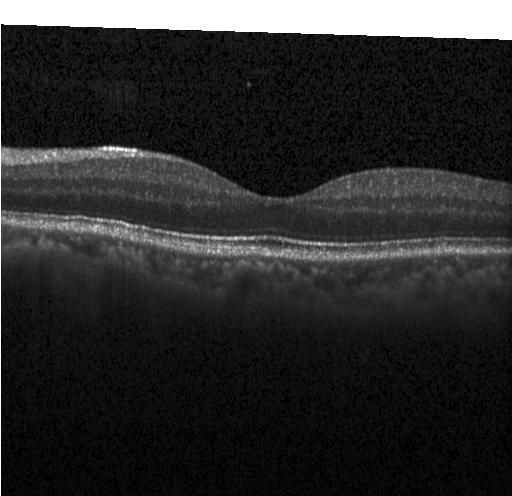 OCT finding: no evidence of choroidal neovascularization, diabetic macular edema, or drusen.